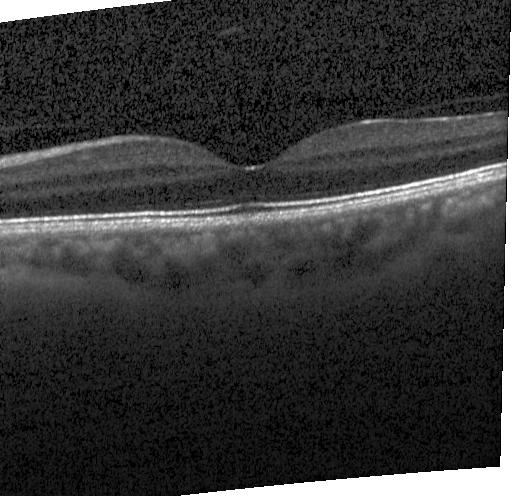
Retinal OCT cross-section · Heidelberg Spectralis · macular scan · spectral-domain optical coherence tomography.
Impression: no CNV, DME, or drusen.